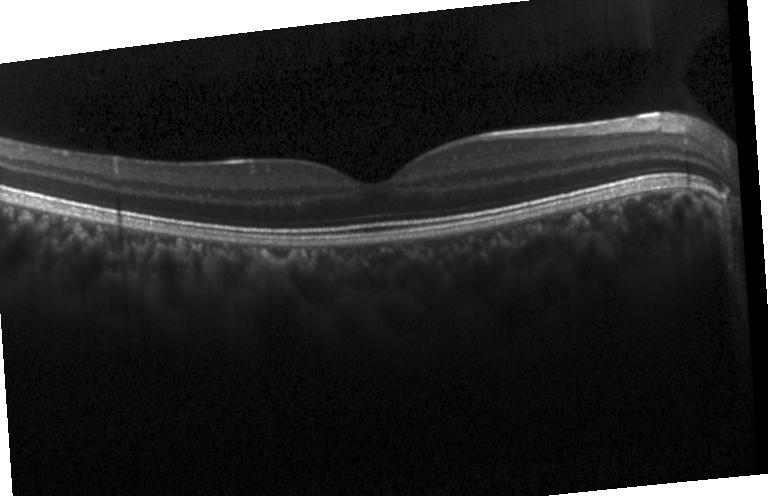
Optical coherence tomography scan
The scan shows no choroidal neovascularization, diabetic macular edema, or drusen.